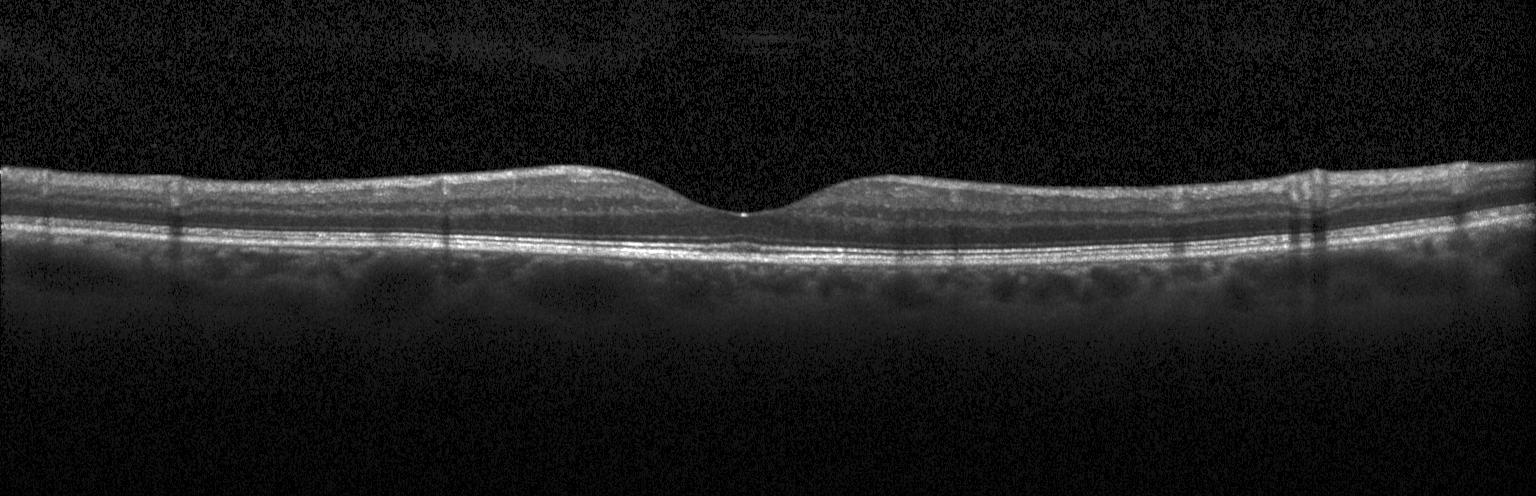 Centered on the fovea. Optical coherence tomography scan. Macular OCT: no CNV, no DME, and no drusen.